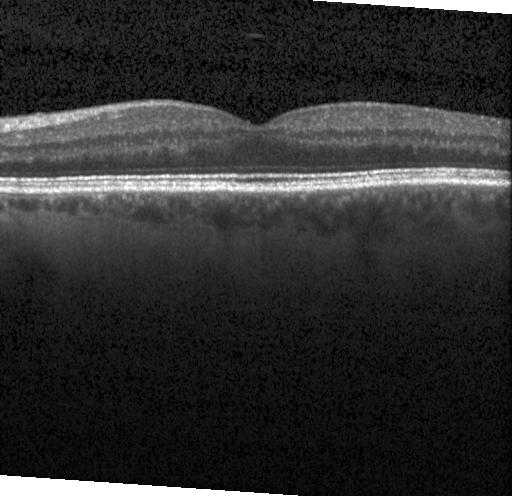 Instrument: Heidelberg Spectralis · through the macula · optical coherence tomography scan
The scan shows no choroidal neovascularization, no diabetic macular edema, and no drusen.